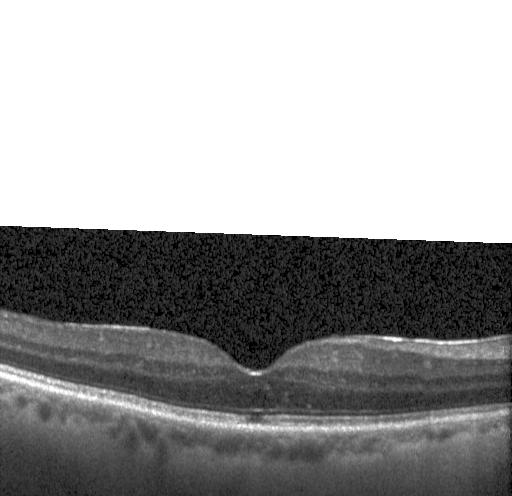
Fovea-centered. Retinal OCT B-scan
Neither choroidal neovascularization, diabetic macular edema, nor drusen.